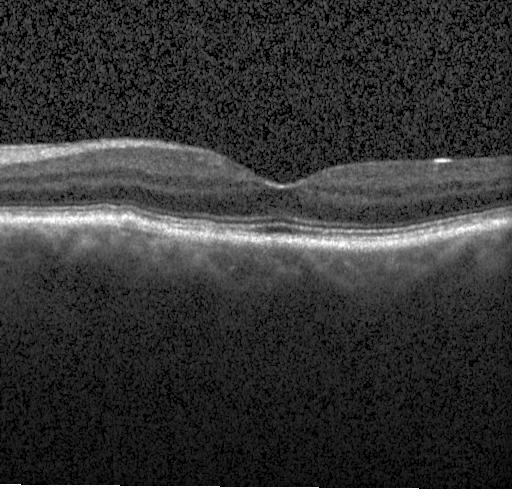 Retinal OCT cross-section · SD-OCT
Finding: multiple drusen.